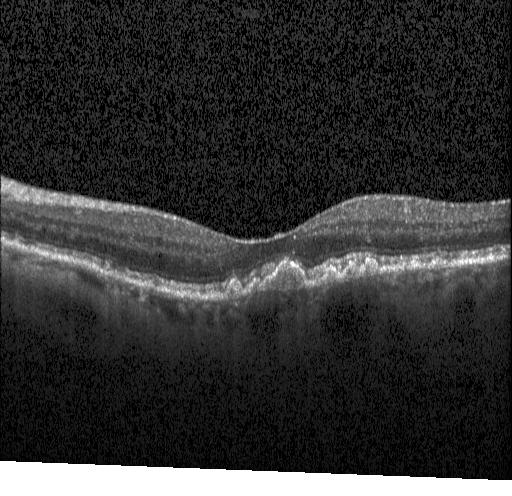 SD-OCT · fovea-centered · retinal OCT cross-section
This B-scan demonstrates multiple drusen.